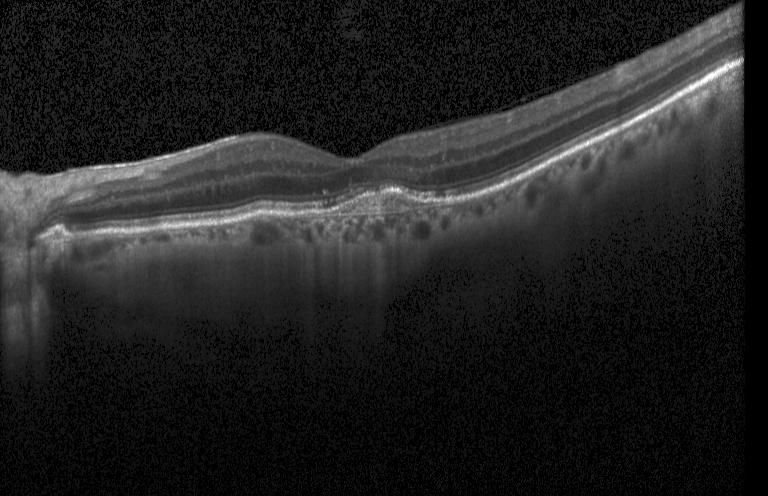 The scan shows choroidal neovascularization (CNV).